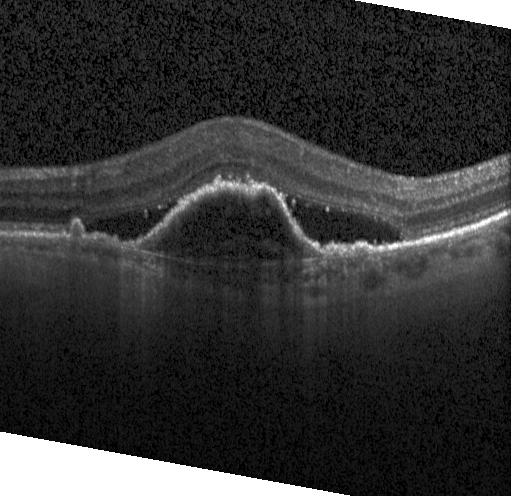
Macular OCT demonstrating choroidal neovascularization (CNV).